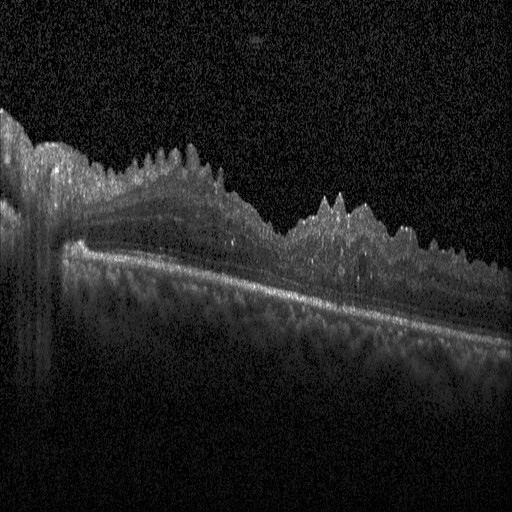 OCT scan showing diabetic macular edema.